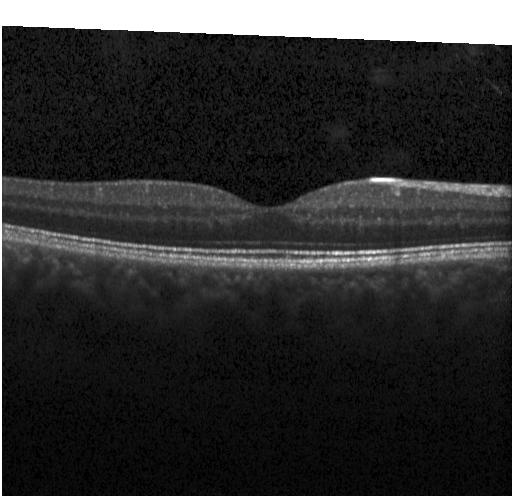

Dx: neither choroidal neovascularization, diabetic macular edema, nor drusen.